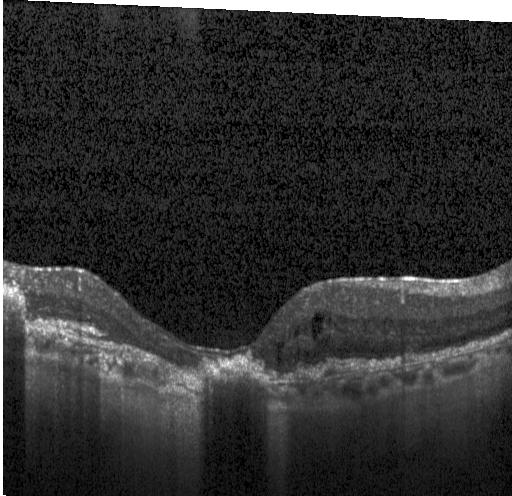 Finding: a choroidal neovascular membrane.